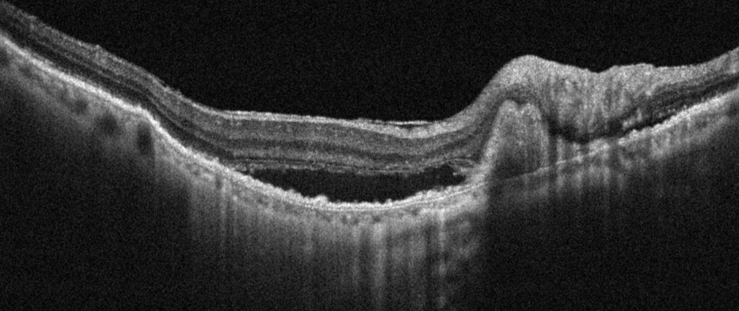
Retinal OCT cross-section showing AMD.